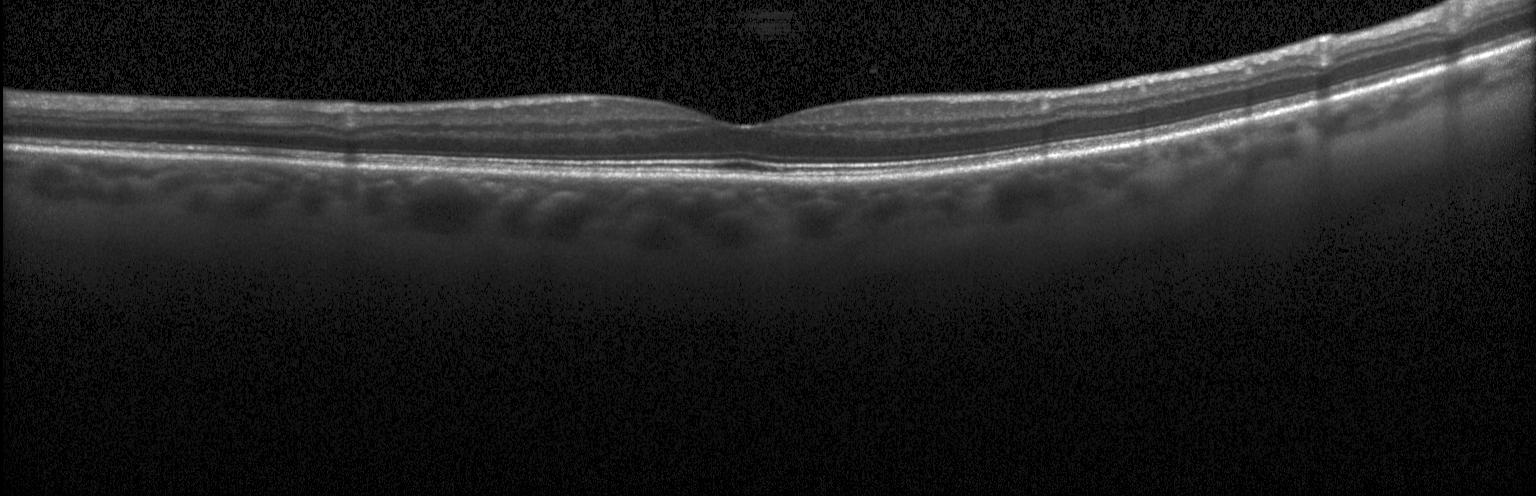
Horizontal scan through the fovea, optical coherence tomography B-scan, SD-OCT. Diagnosis: no evidence of choroidal neovascularization, diabetic macular edema, or drusen.